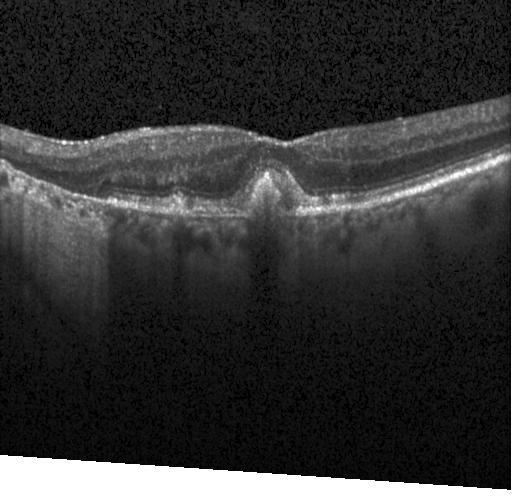

Fovea-centered · OCT B-scan · instrument: Heidelberg Spectralis · SD-OCT.
Finding: a choroidal neovascular membrane.